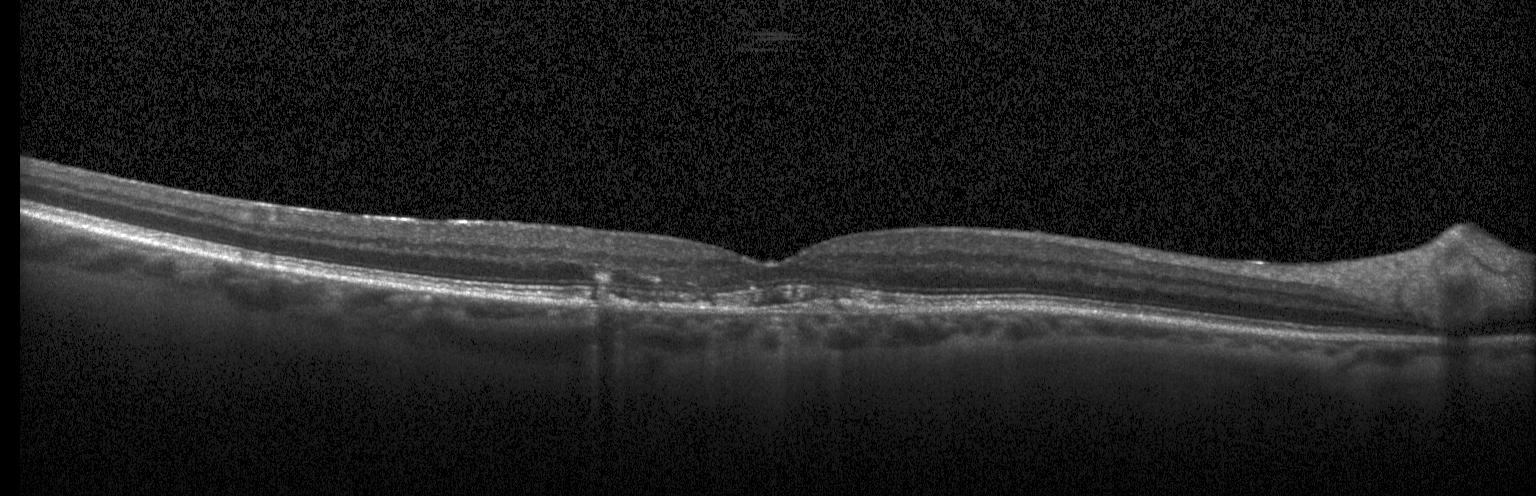

This B-scan demonstrates choroidal neovascularization.